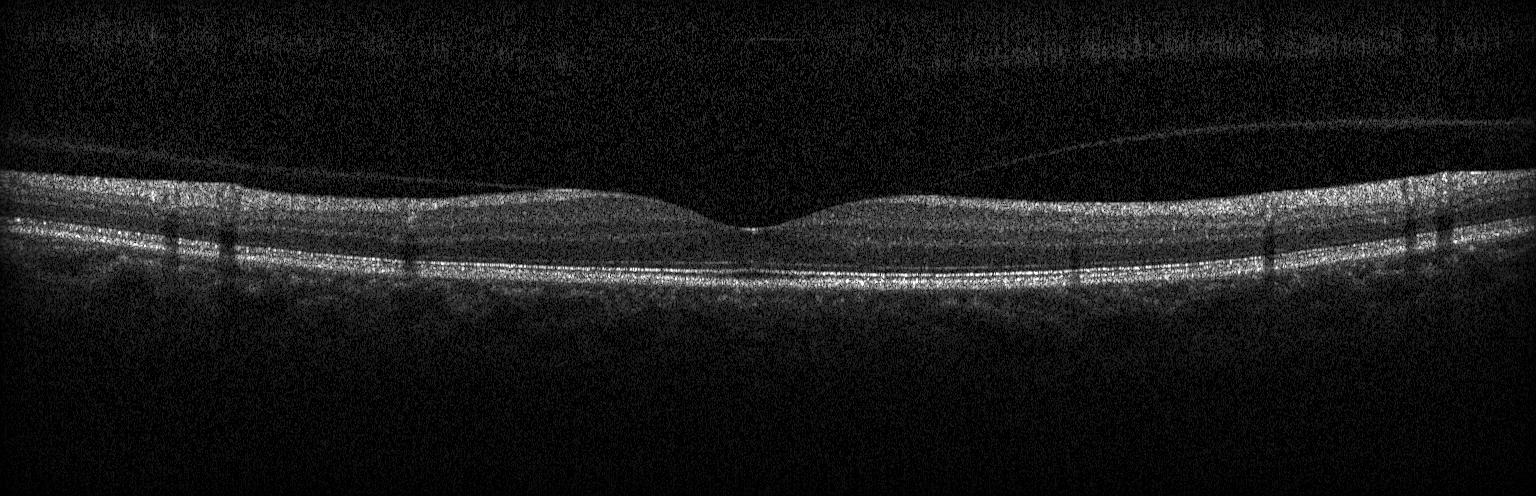 Finding: no choroidal neovascularization, no diabetic macular edema, and no drusen.